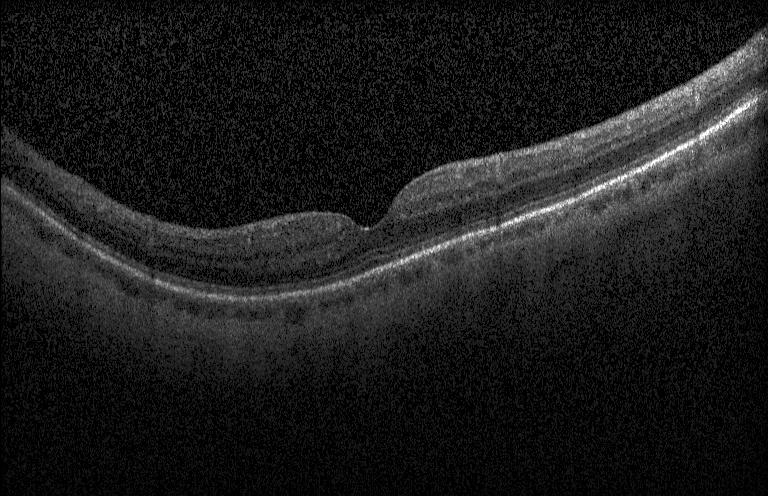

Optical coherence tomography B-scan · SD-OCT. Dx: no evidence of CNV, DME, or drusen.